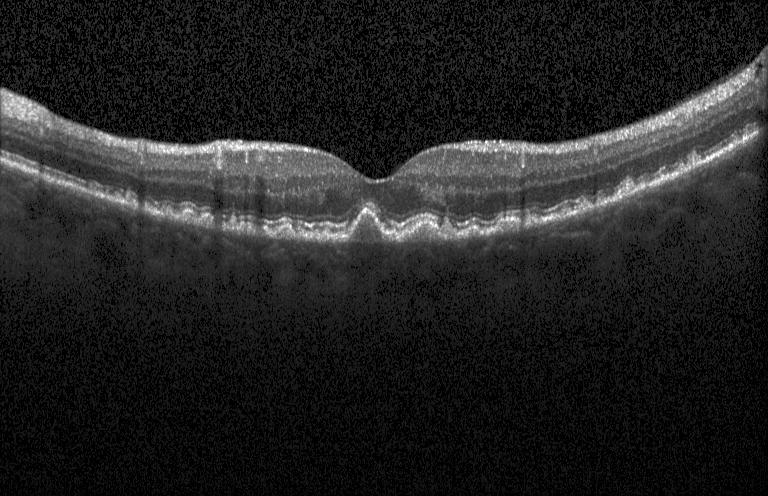
Dx: sub-RPE drusenoid deposits.